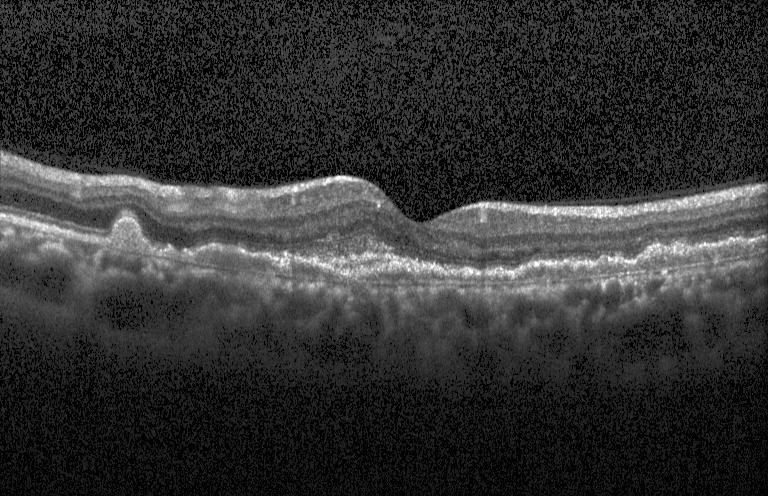 OCT line scan
This B-scan demonstrates a choroidal neovascular membrane.